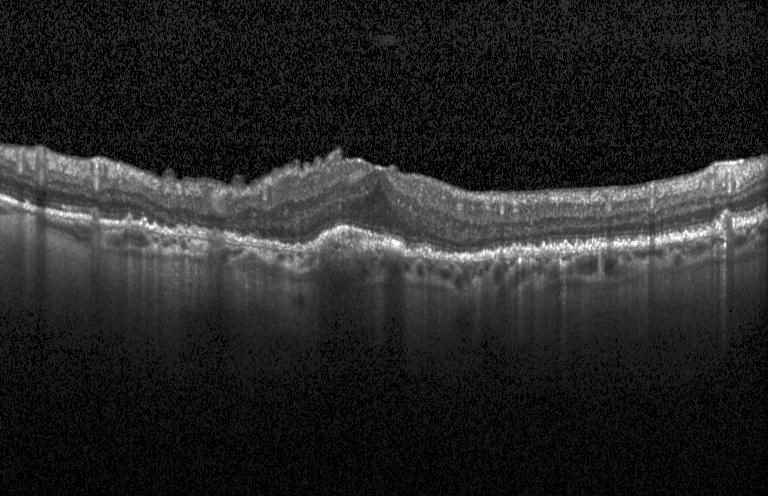
Assessment: CNV.